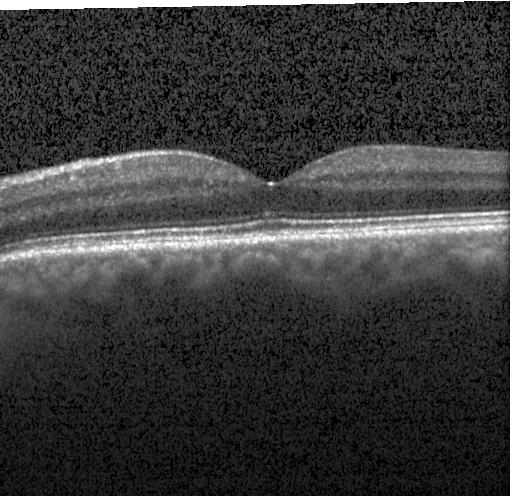

Instrument: Heidelberg Spectralis. Through the macula. Spectral-domain OCT. Optical coherence tomography scan
Diagnosis: no CNV, no DME, and no drusen.